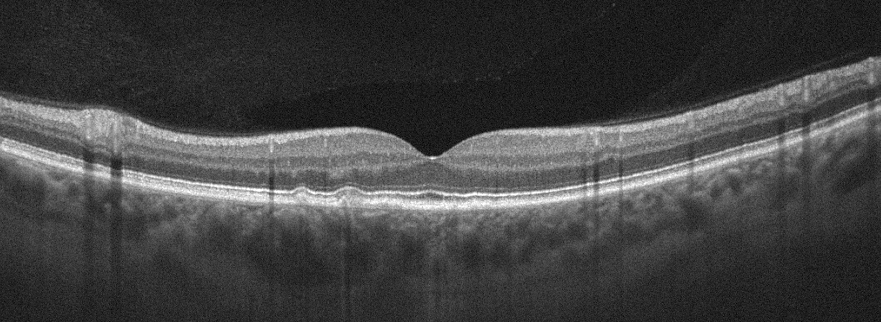
Oculus sinister · optical coherence tomography scan. OCT finding: age-related macular degeneration (AMD).